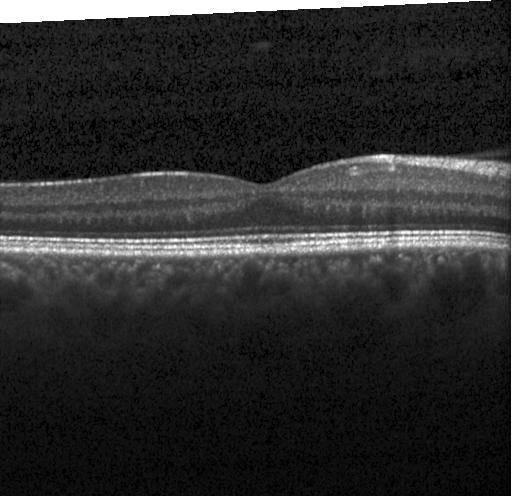

Impression: neither choroidal neovascularization, diabetic macular edema, nor drusen.